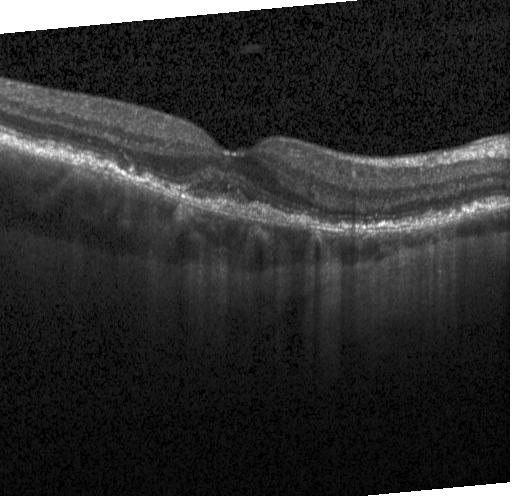 Dx: choroidal neovascularization.